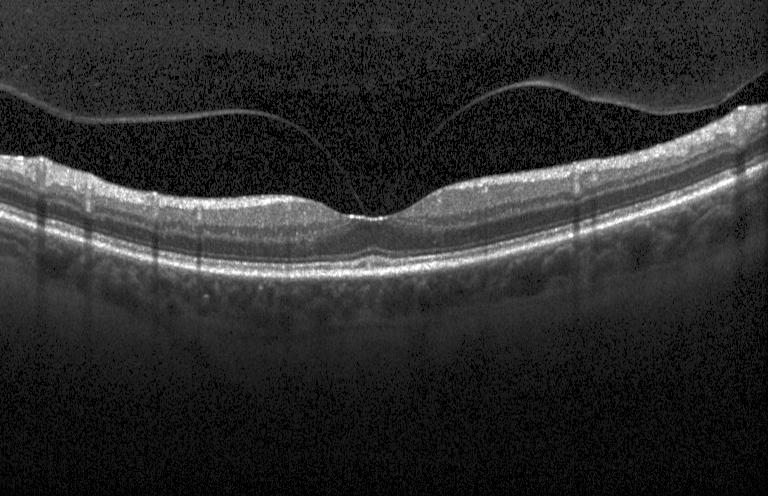
Heidelberg Spectralis. Centered on the fovea. Spectral-domain OCT. Optical coherence tomography B-scan.
This B-scan demonstrates no choroidal neovascularization, diabetic macular edema, or drusen.